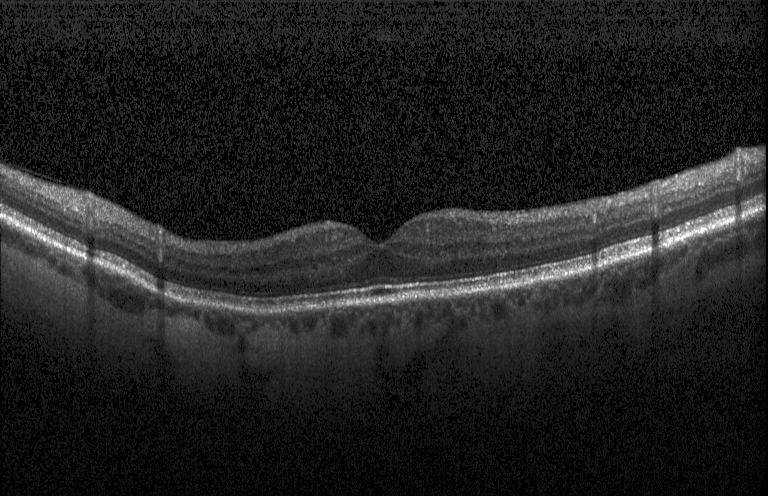

Macular OCT demonstrating no choroidal neovascularization, no diabetic macular edema, and no drusen.